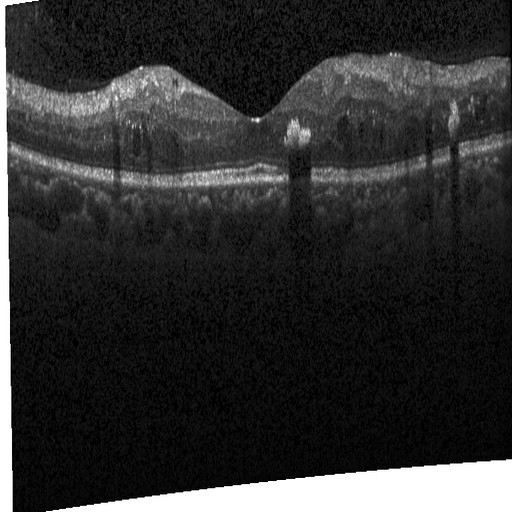

Fovea-centered · acquired on a Heidelberg Spectralis · retinal OCT cross-section · spectral-domain OCT. Macular OCT: diabetic macular edema.